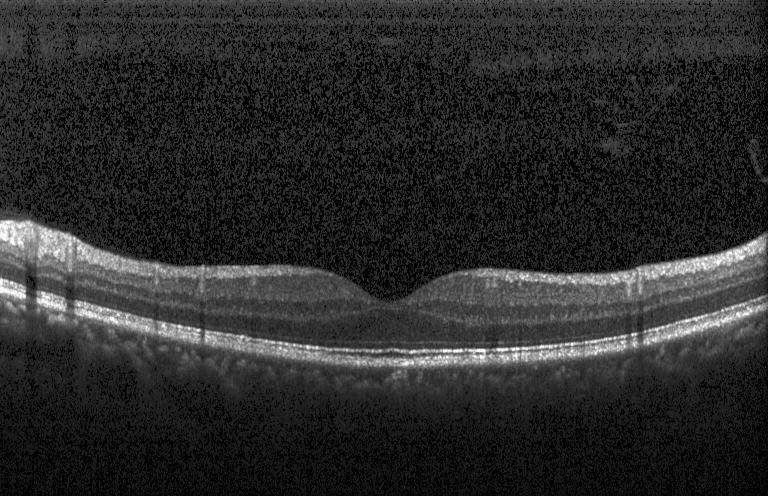

No choroidal neovascularization, no diabetic macular edema, and no drusen.